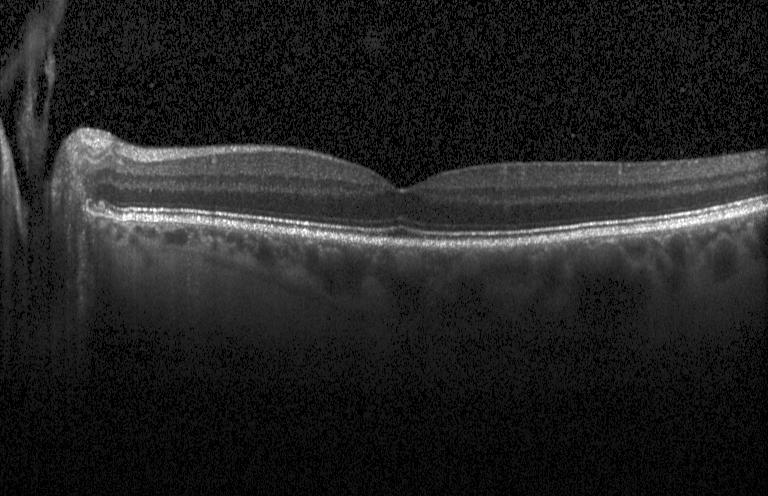 Optical coherence tomography scan. Dx: no CNV, no DME, and no drusen.